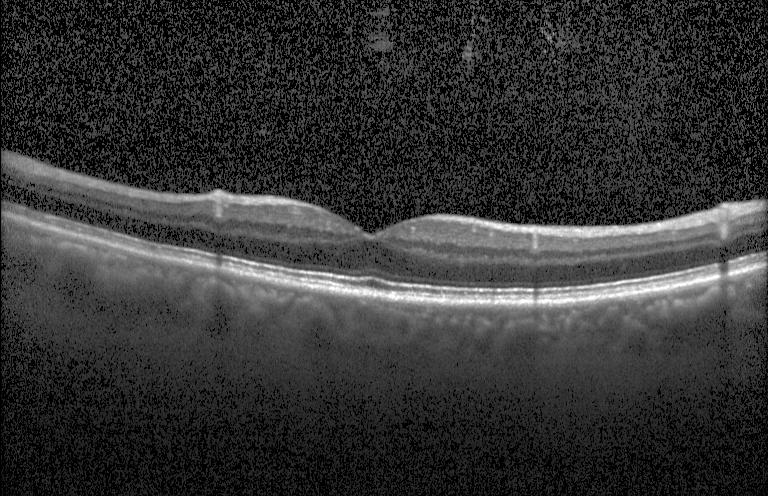 Heidelberg Spectralis. Centered on the fovea. Retinal OCT cross-section
OCT finding: no CNV, DME, or drusen.